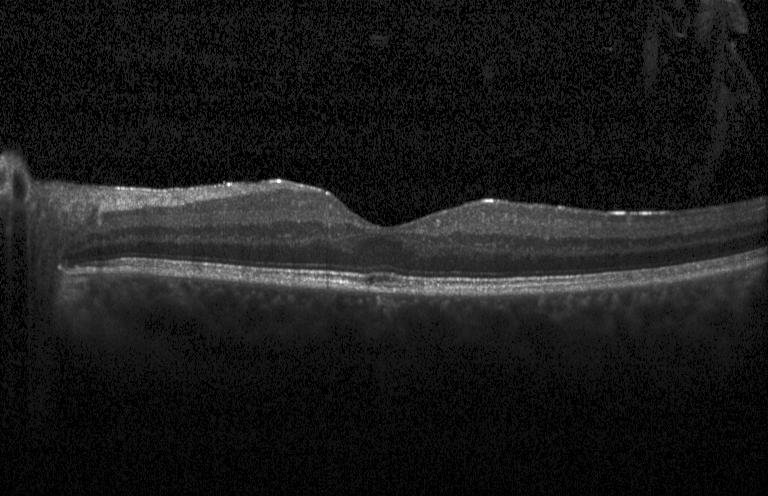

SD-OCT. Retinal OCT B-scan
Dx: no CNV, no DME, and no drusen.